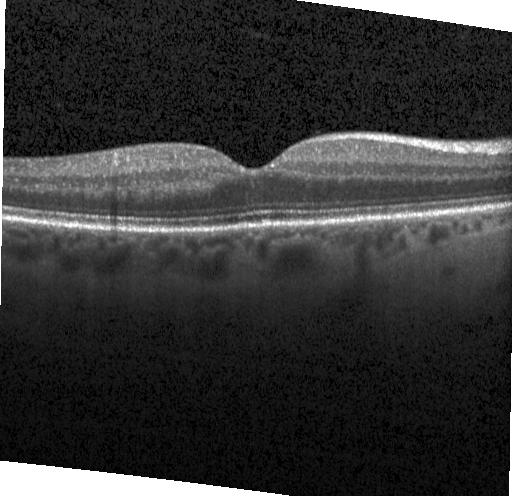

Optical coherence tomography B-scan — Impression: no CNV, no DME, and no drusen.